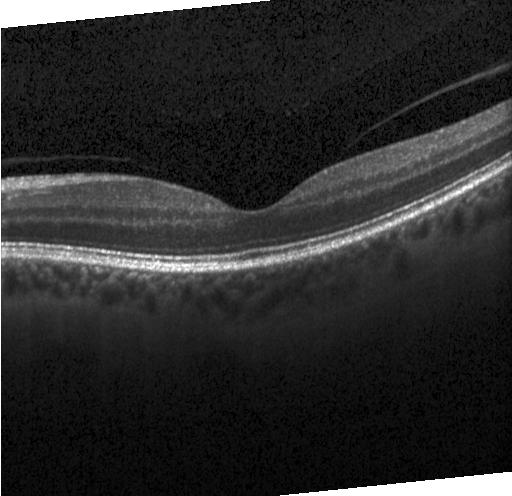 Centered on the fovea. Acquired on a Heidelberg Spectralis. Optical coherence tomography B-scan
Impression: no choroidal neovascularization, no diabetic macular edema, and no drusen.